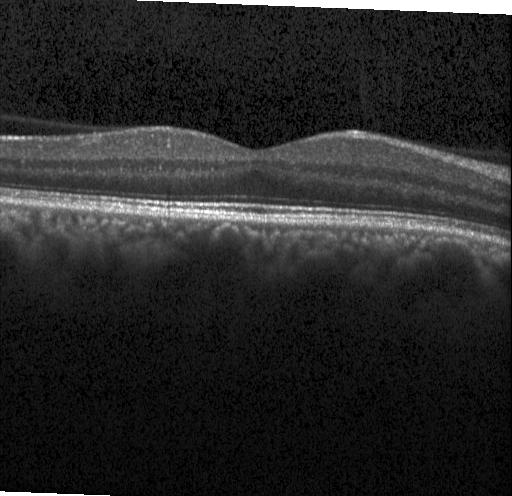 Finding: neither choroidal neovascularization, diabetic macular edema, nor drusen.